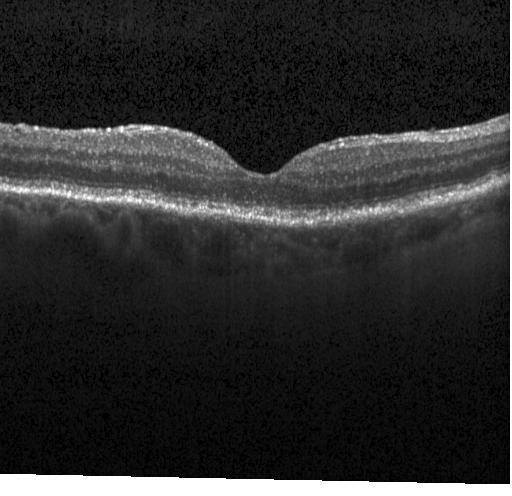
OCT B-scan · instrument: Heidelberg Spectralis.
Assessment: no CNV, no DME, and no drusen.